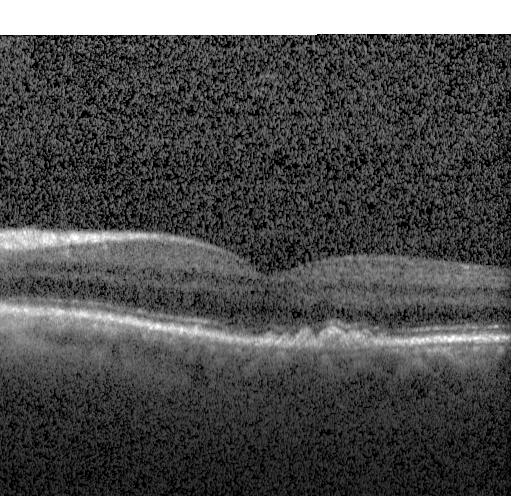
Retinal OCT cross-section, horizontal scan through the fovea. Macular OCT: multiple drusen.